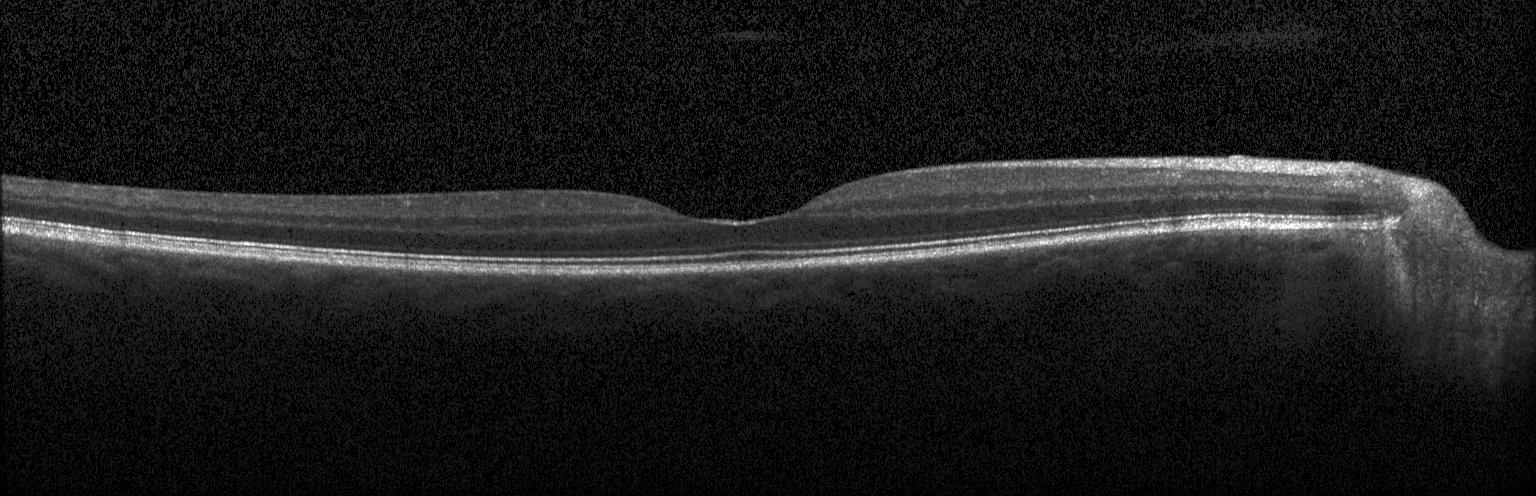 Spectral-domain OCT, retinal OCT cross-section
Impression: neither choroidal neovascularization, diabetic macular edema, nor drusen.